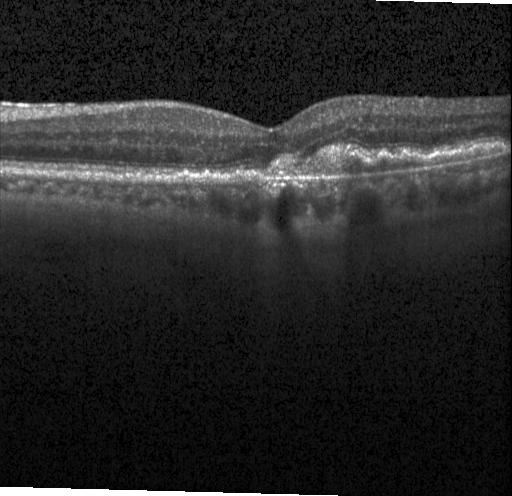

OCT B-scan. Spectral-domain optical coherence tomography. Fovea-centered.
Assessment: choroidal neovascularization (CNV).